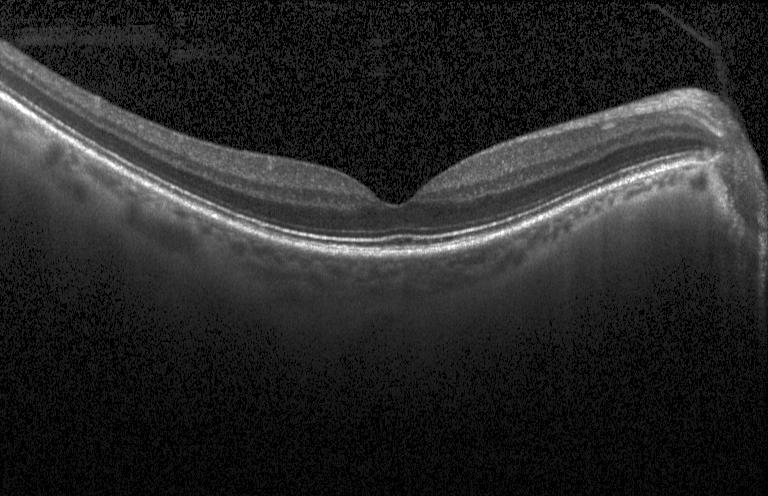
Optical coherence tomography B-scan · horizontal scan through the fovea · Heidelberg Spectralis OCT system · spectral-domain optical coherence tomography — Macular OCT: no choroidal neovascularization, diabetic macular edema, or drusen.